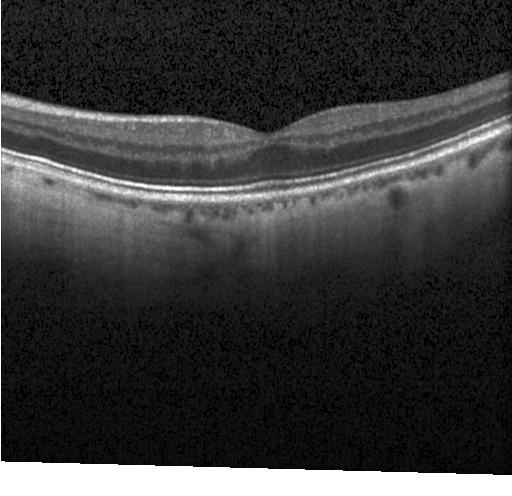 Optical coherence tomography scan. Horizontal scan through the fovea. Impression: no evidence of CNV, DME, or drusen.